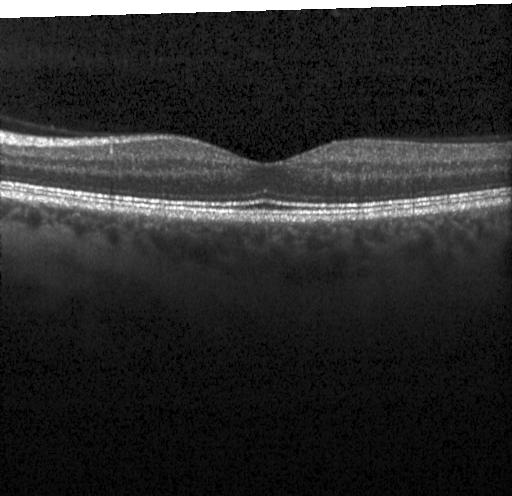
Finding: no evidence of choroidal neovascularization, diabetic macular edema, or drusen.